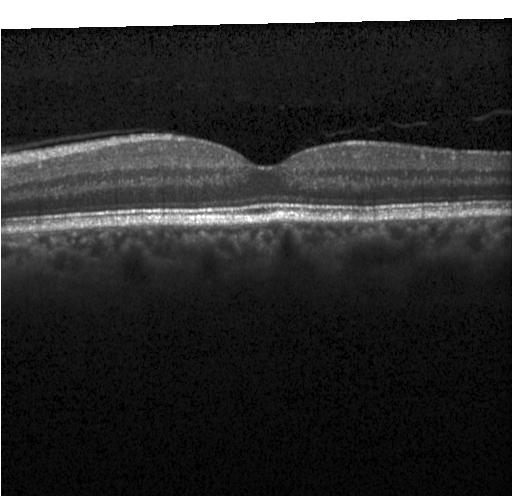 Optical coherence tomography scan, Heidelberg Spectralis, SD-OCT
Diagnosis: no choroidal neovascularization, diabetic macular edema, or drusen.